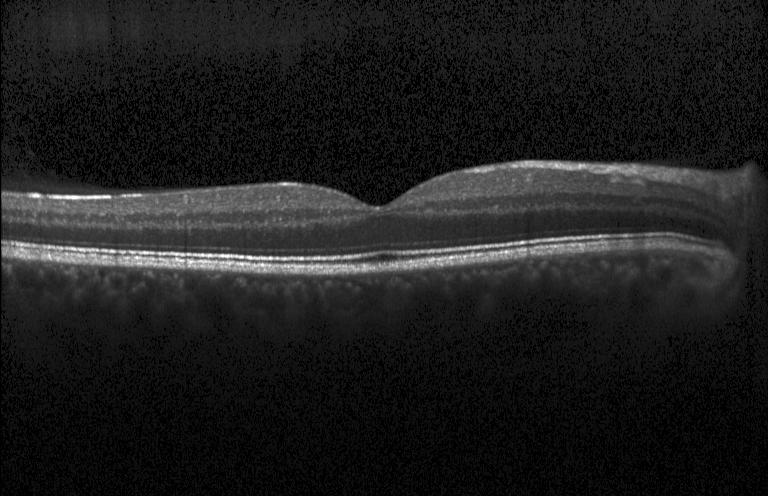

Optical coherence tomography B-scan · SD-OCT · Heidelberg Spectralis
Finding: neither choroidal neovascularization, diabetic macular edema, nor drusen.